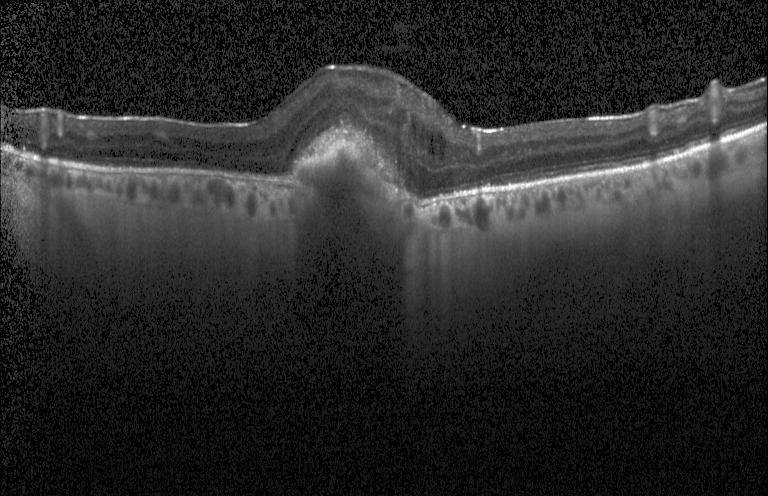 Retinal OCT cross-section — The scan shows choroidal neovascularization (CNV).